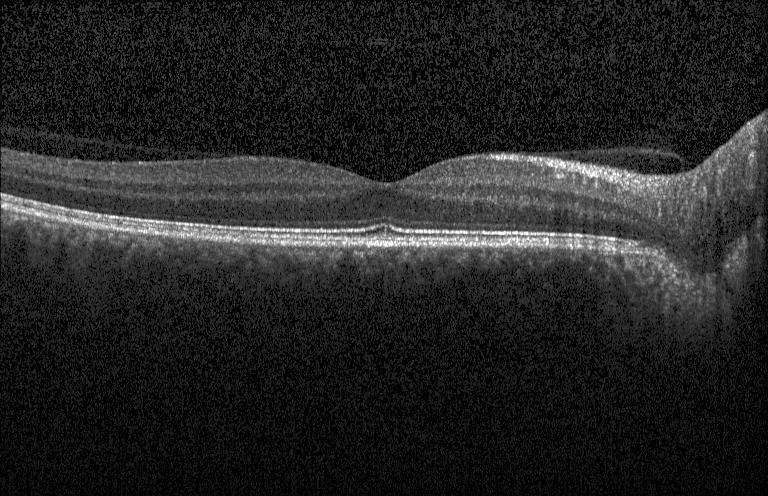 OCT line scan.
Impression: neither choroidal neovascularization, diabetic macular edema, nor drusen.